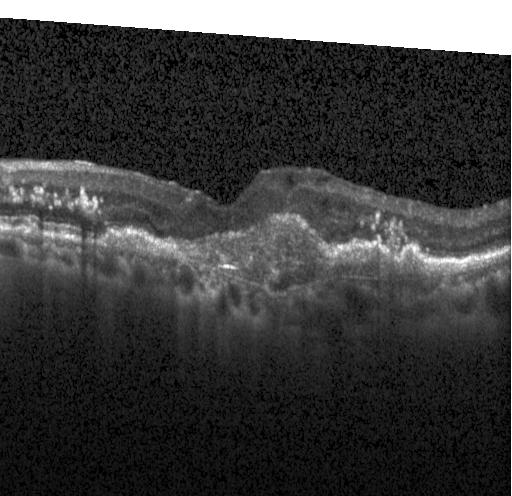

Acquired on a Heidelberg Spectralis. Optical coherence tomography scan
OCT finding: a choroidal neovascular membrane.